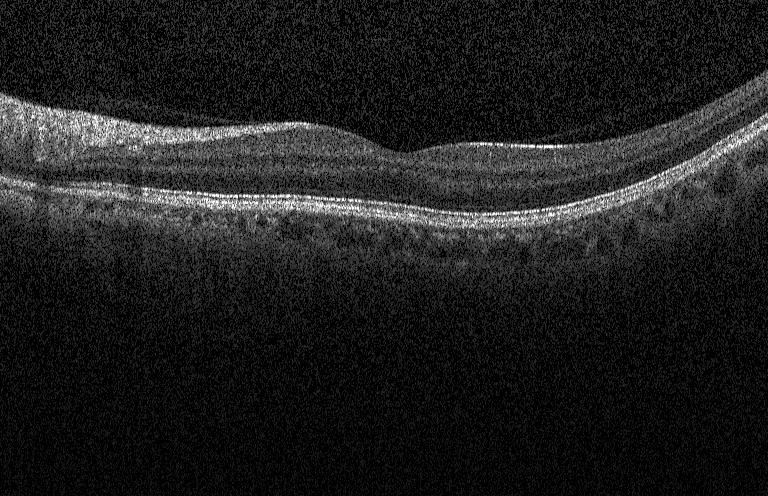 Retinal OCT B-scan — No choroidal neovascularization, diabetic macular edema, or drusen.